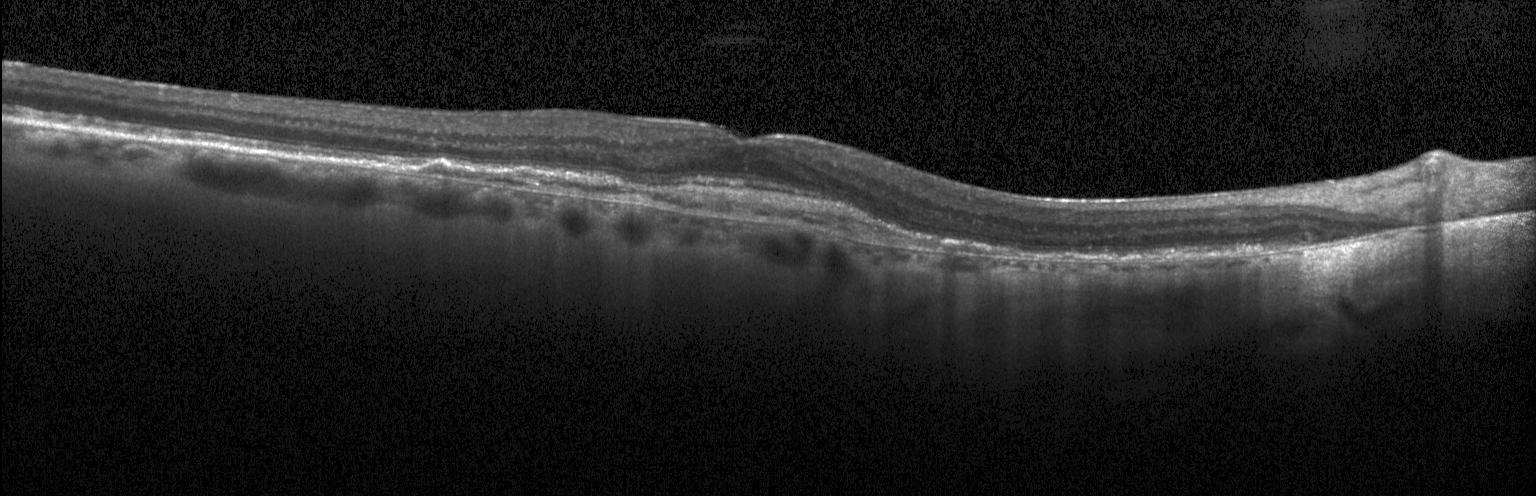

Retinal OCT cross-section, fovea-centered
Diagnosis: CNV.